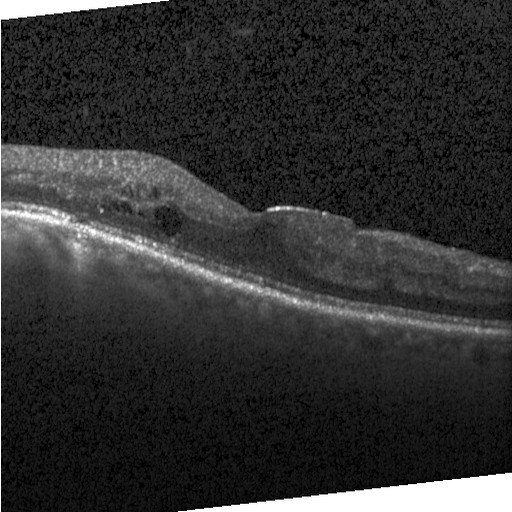
Heidelberg Spectralis OCT system; centered on the fovea; spectral-domain OCT; OCT B-scan.
This B-scan demonstrates DME.